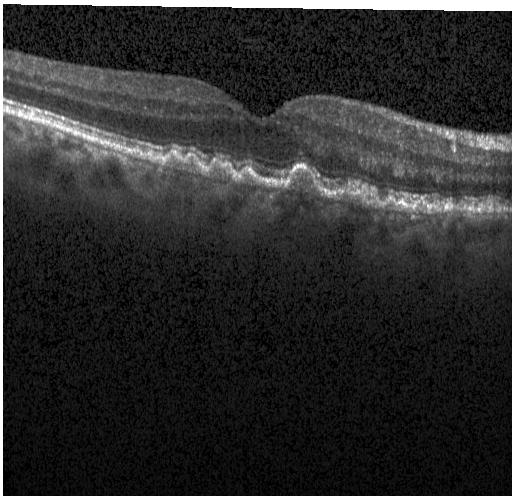
Retinal OCT B-scan
Diagnosis: multiple drusen.